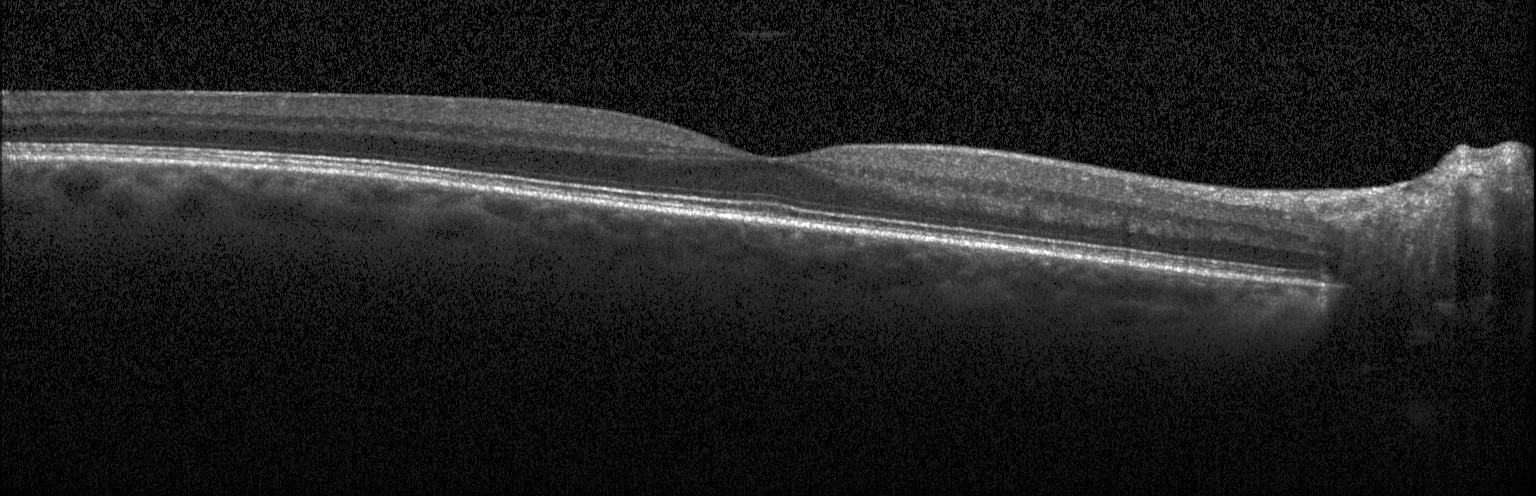
Macular OCT demonstrating neither choroidal neovascularization, diabetic macular edema, nor drusen.